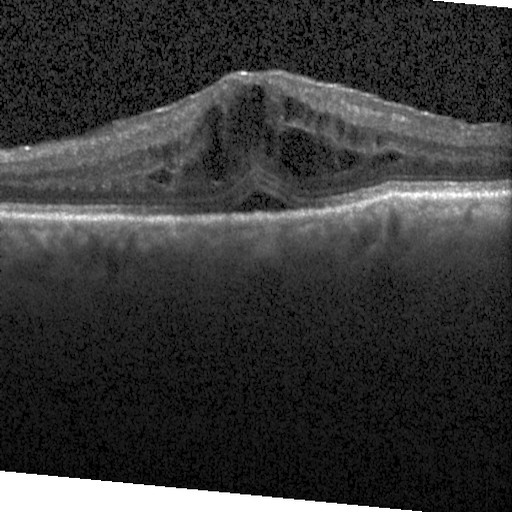
Assessment: diabetic macular edema.